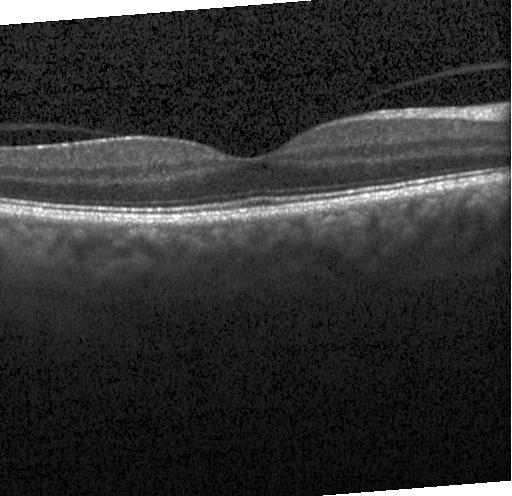

Heidelberg Spectralis OCT system. Optical coherence tomography scan
This B-scan demonstrates no choroidal neovascularization, diabetic macular edema, or drusen.